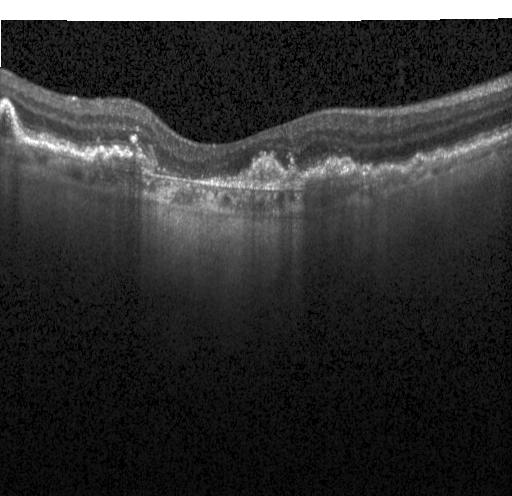
Spectral-domain OCT. Through the macula. Heidelberg Spectralis. OCT line scan. This B-scan demonstrates choroidal neovascularization.